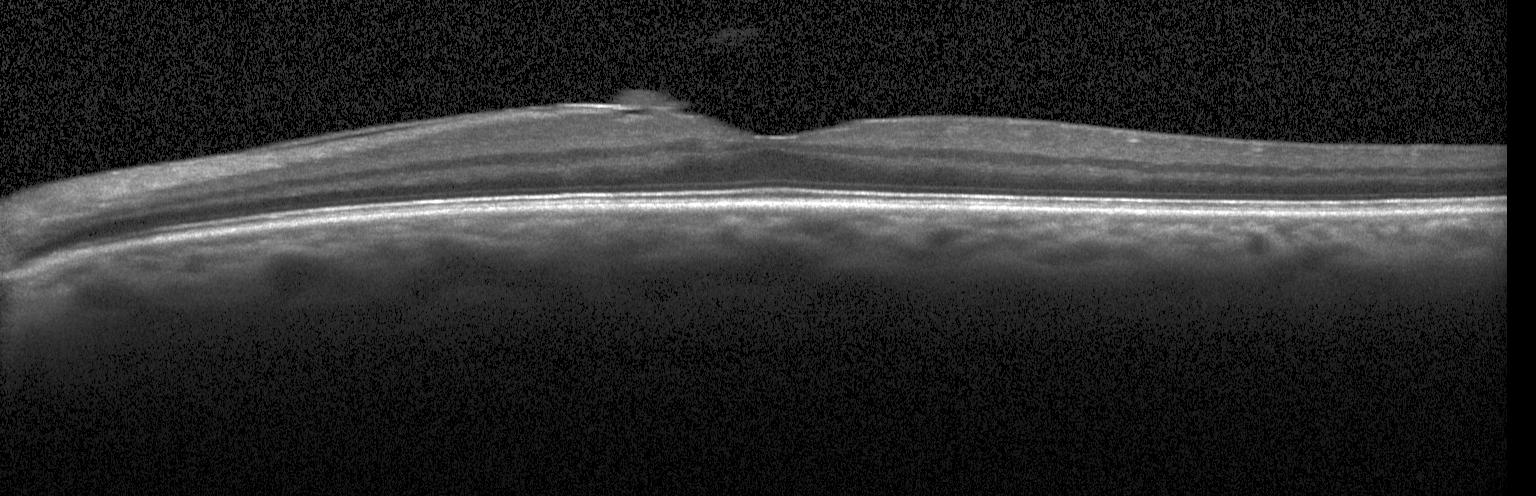

Retinal OCT cross-section.
Impression: neither CNV, DME, nor drusen.